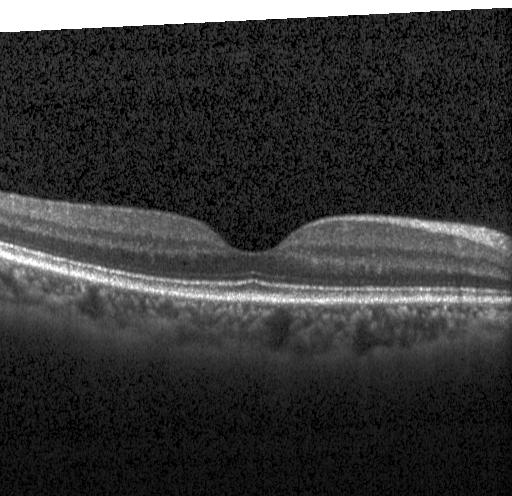
Retinal OCT cross-section showing no evidence of choroidal neovascularization, diabetic macular edema, or drusen.